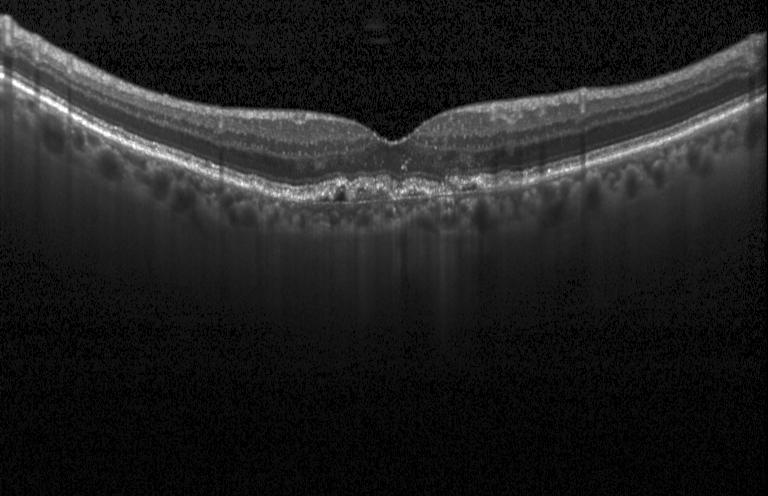

OCT B-scan; Heidelberg Spectralis — OCT finding: choroidal neovascularization (CNV).